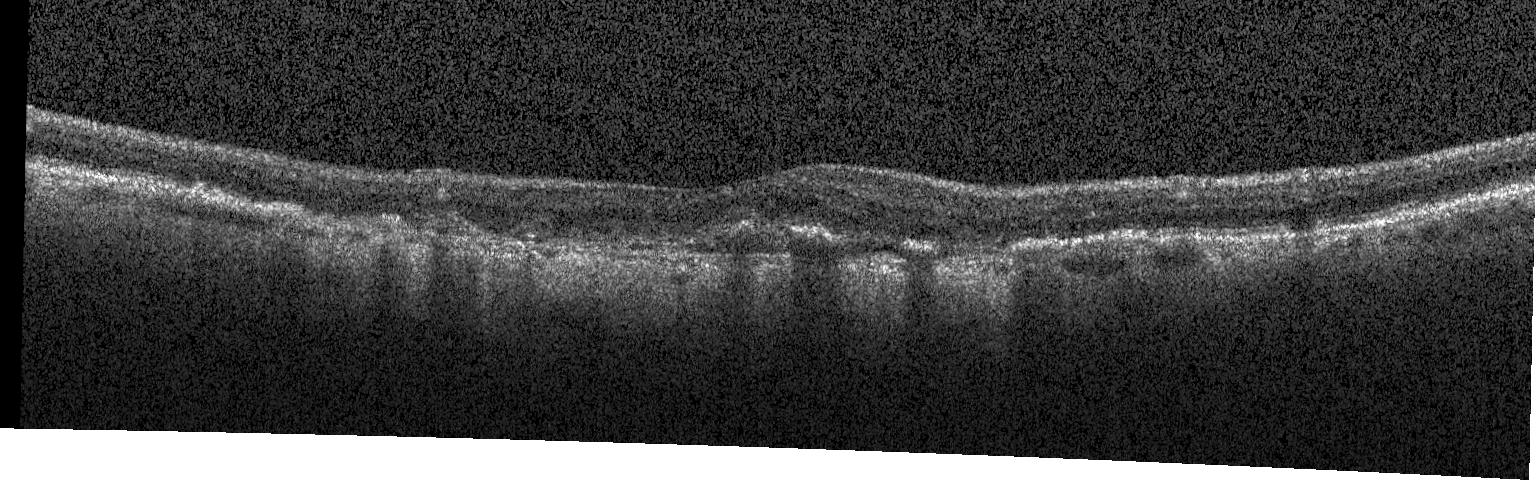
OCT B-scan. Acquired on a Heidelberg Spectralis. Spectral-domain optical coherence tomography. Horizontal scan through the fovea — Assessment: a choroidal neovascular membrane.